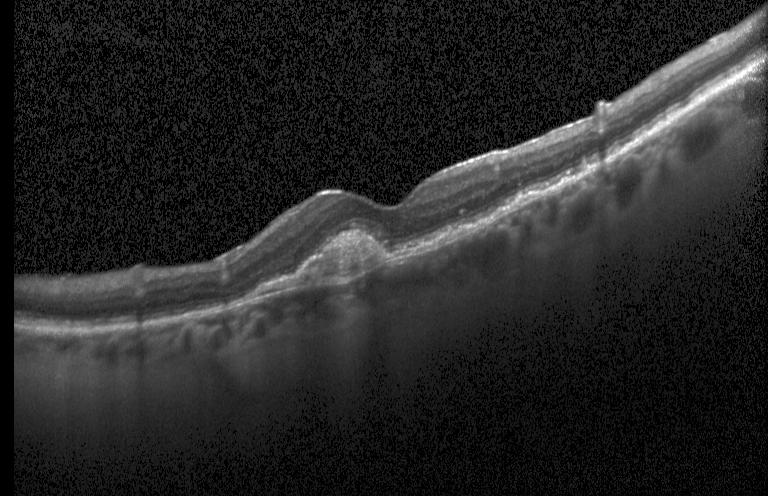

SD-OCT. Fovea-centered. Optical coherence tomography scan. Heidelberg Spectralis OCT system. Choroidal neovascularization (CNV).